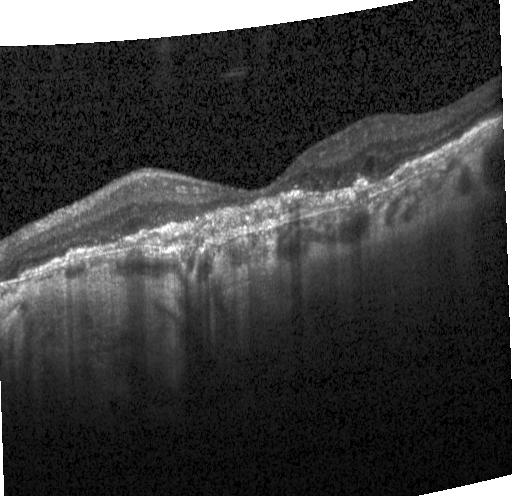

Optical coherence tomography B-scan.
Diagnosis: choroidal neovascularization (CNV).